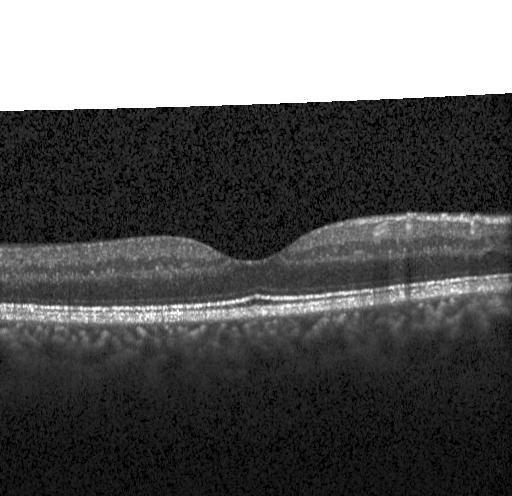

Diagnosis: no CNV, no DME, and no drusen.